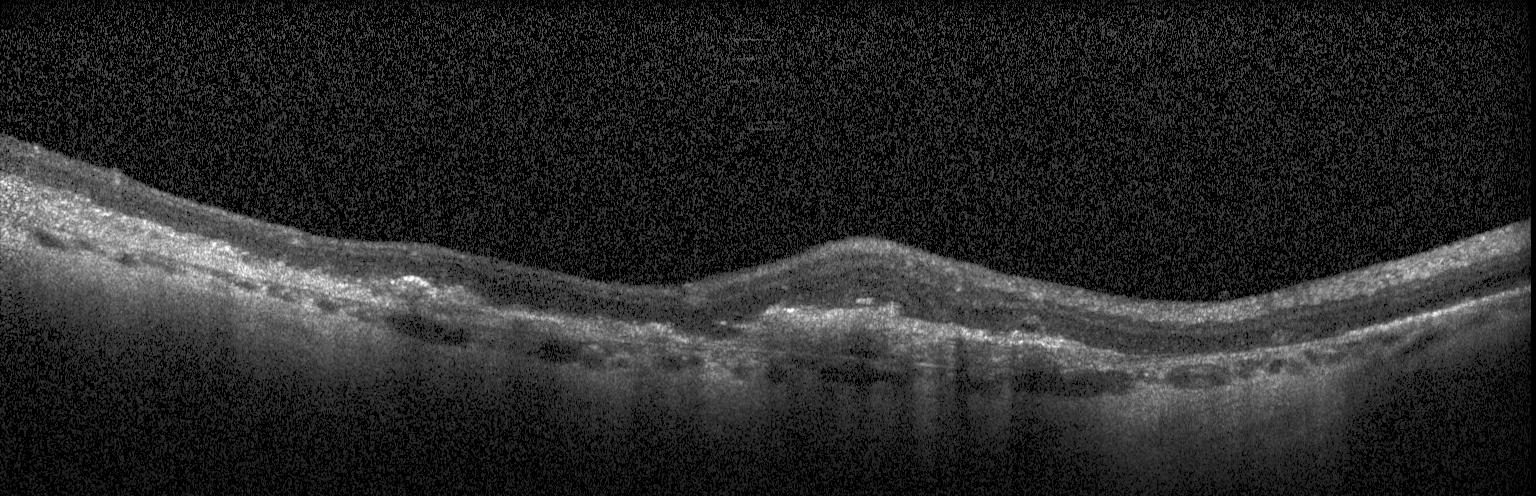 Retinal OCT B-scan, instrument: Heidelberg Spectralis, fovea-centered — Finding: choroidal neovascularization (CNV).